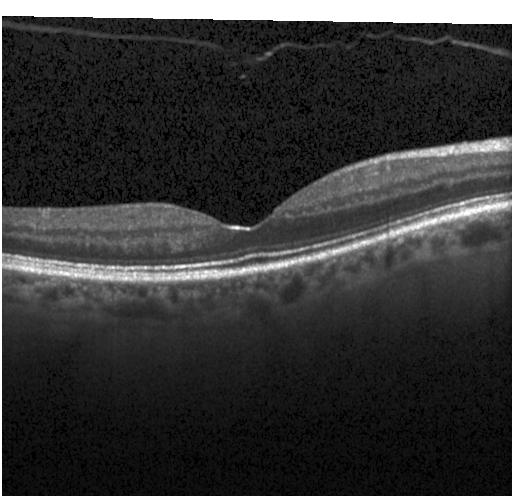 Neither choroidal neovascularization, diabetic macular edema, nor drusen.